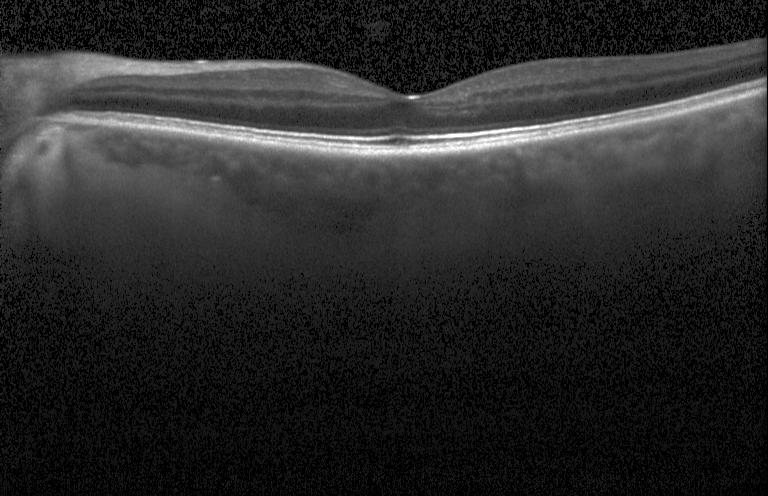 Macular OCT: no CNV, no DME, and no drusen.